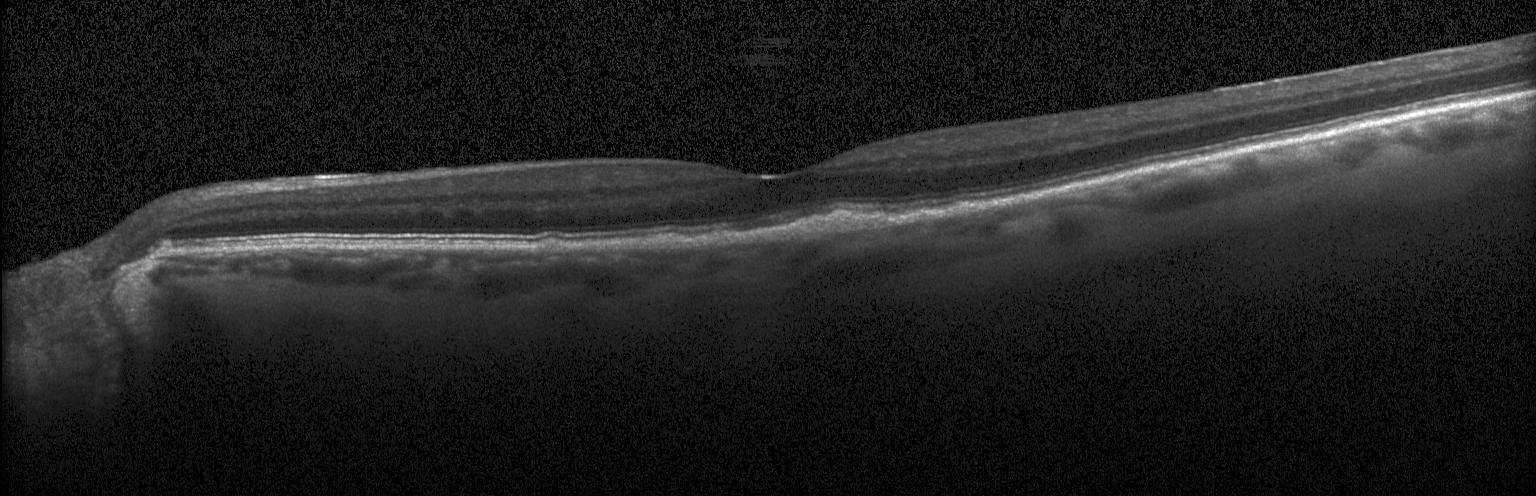
Centered on the fovea; retinal OCT cross-section; spectral-domain optical coherence tomography.
Impression: multiple drusen.